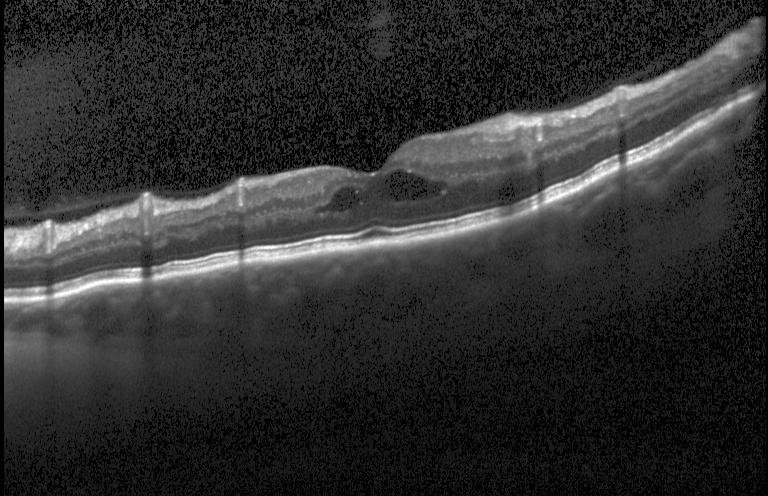 Macular OCT: diabetic macular edema.